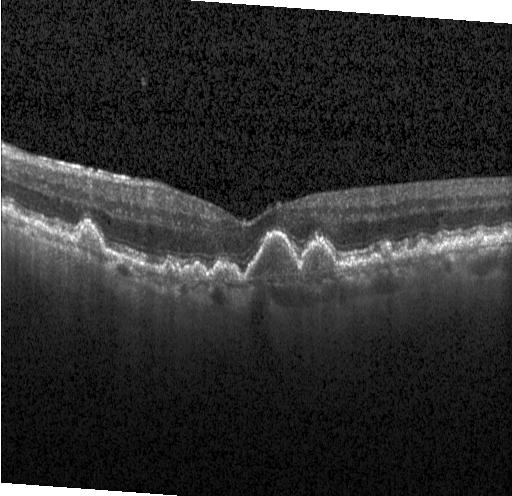

Instrument: Heidelberg Spectralis; horizontal scan through the fovea; spectral-domain optical coherence tomography; OCT line scan.
This B-scan demonstrates multiple drusen.